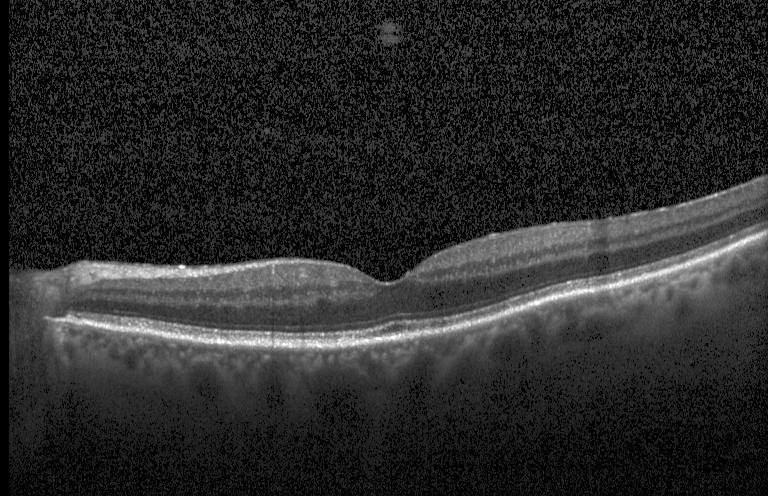
Optical coherence tomography B-scan
Macular OCT: no evidence of CNV, DME, or drusen.